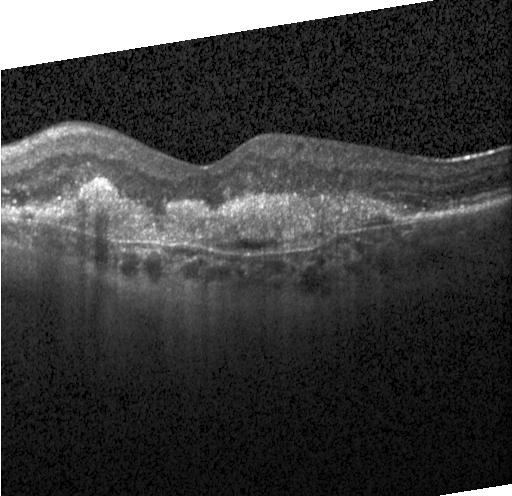

Finding: a choroidal neovascular membrane.